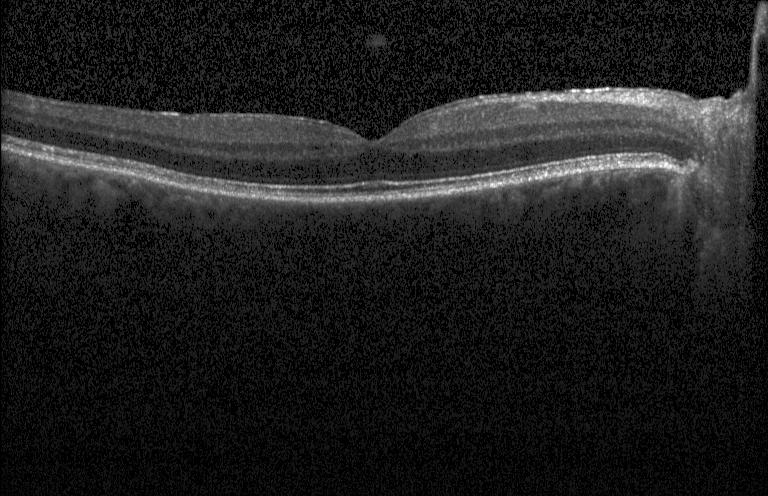
Optical coherence tomography scan — OCT finding: no evidence of choroidal neovascularization, diabetic macular edema, or drusen.